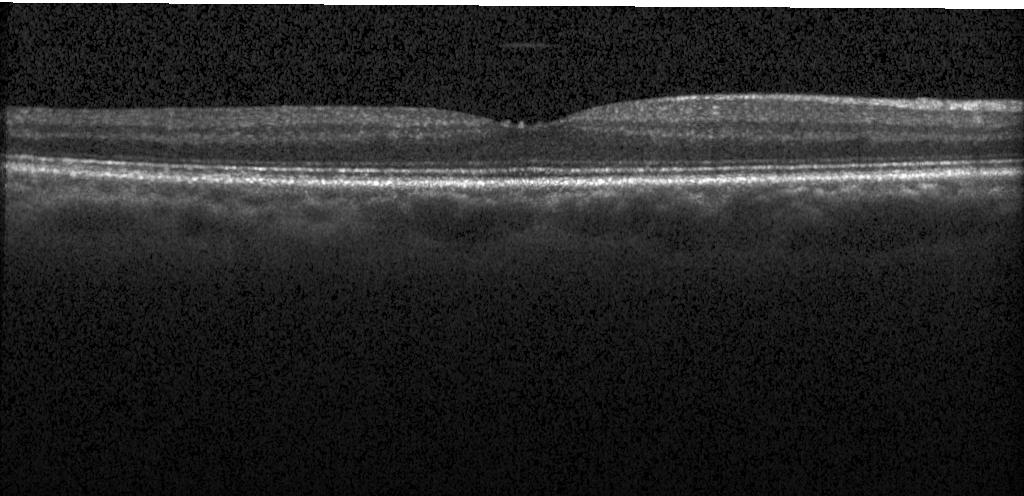
OCT B-scan showing no CNV, DME, or drusen.